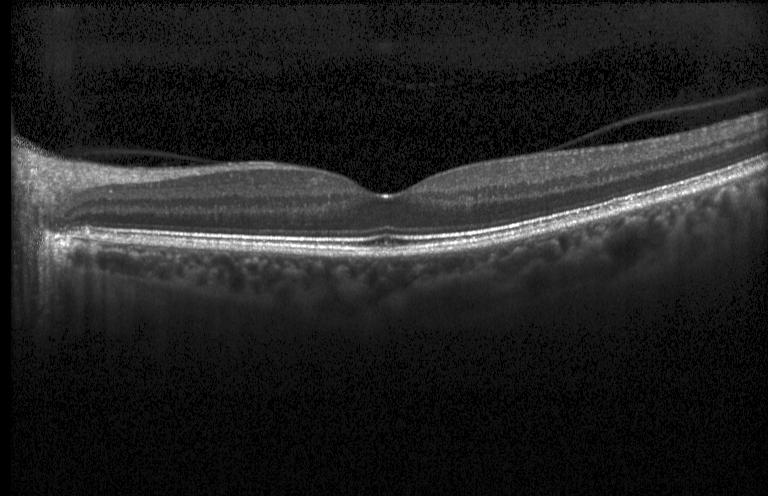
Optical coherence tomography scan; fovea-centered.
This B-scan demonstrates no evidence of CNV, DME, or drusen.